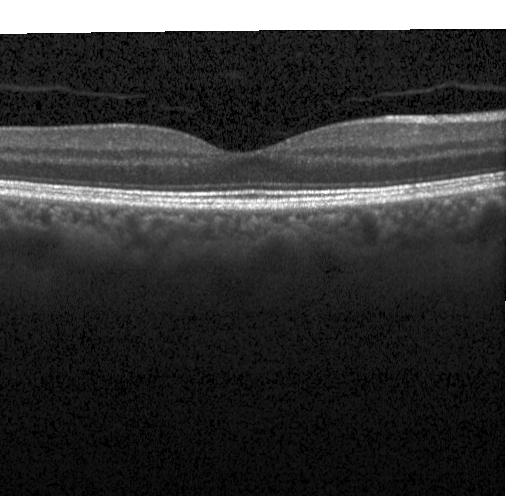
OCT finding: no evidence of CNV, DME, or drusen.